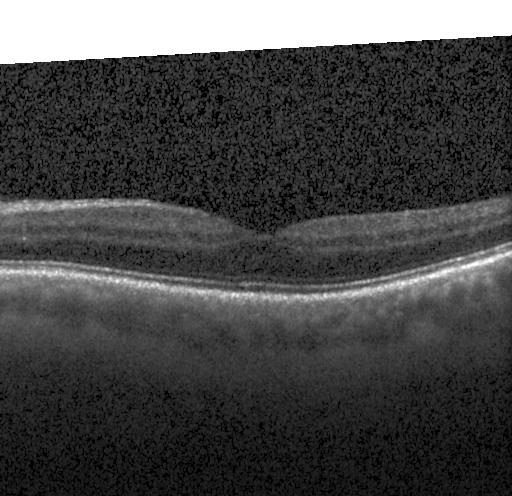
The scan shows no evidence of choroidal neovascularization, diabetic macular edema, or drusen.